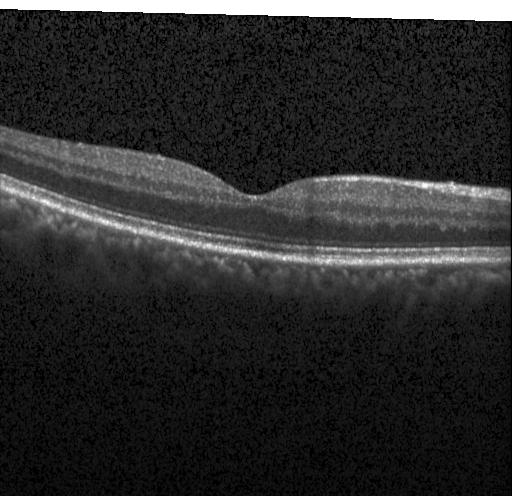

Impression: no CNV, no DME, and no drusen.